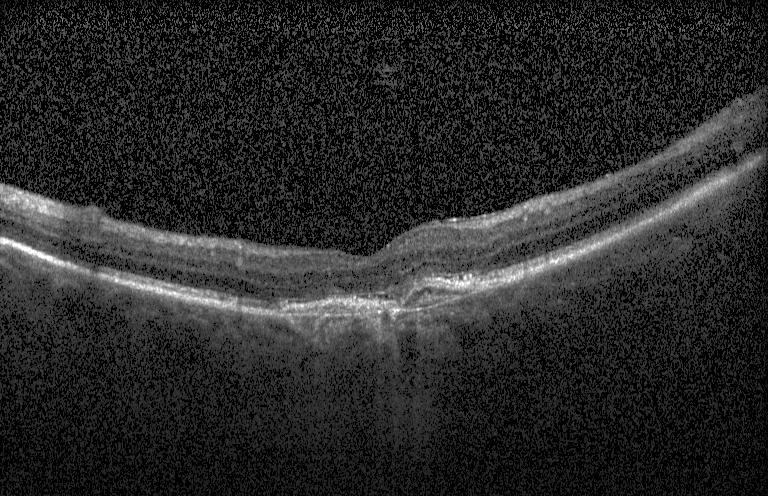

Retinal OCT cross-section. Assessment: choroidal neovascularization (CNV).